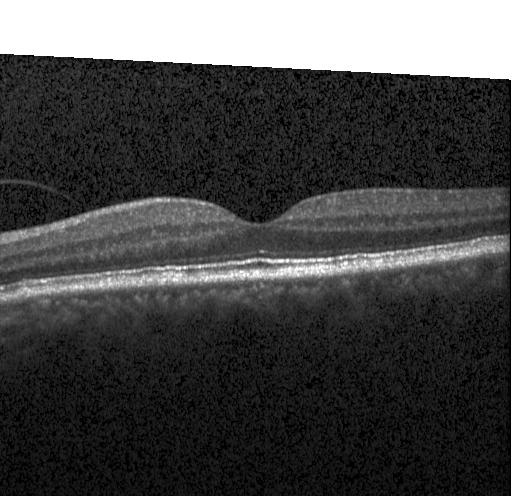 Optical coherence tomography B-scan. OCT finding: no CNV, DME, or drusen.